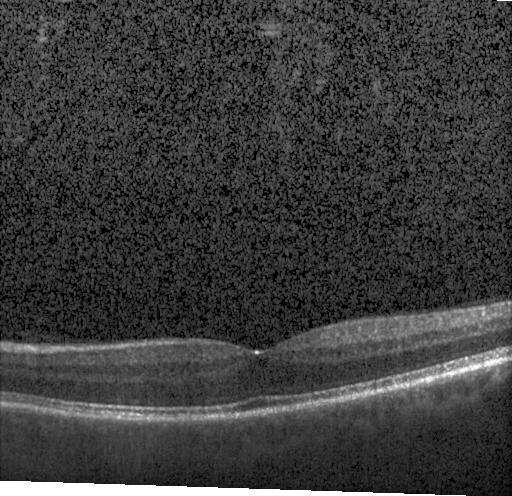

Impression: neither choroidal neovascularization, diabetic macular edema, nor drusen.